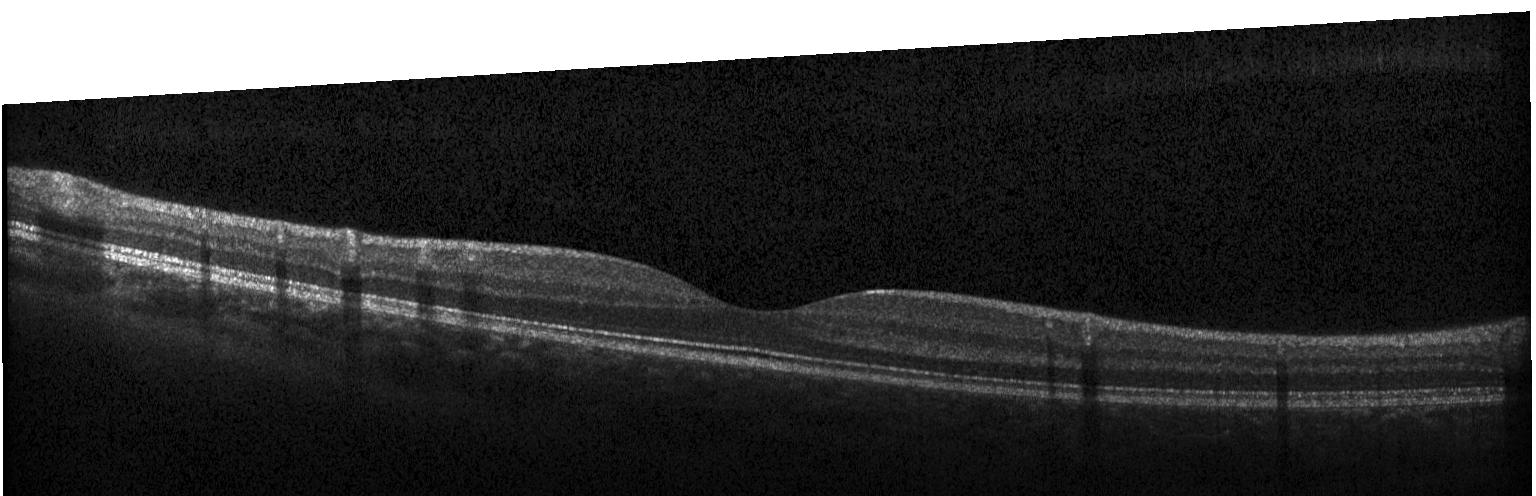
OCT B-scan showing no CNV, DME, or drusen.